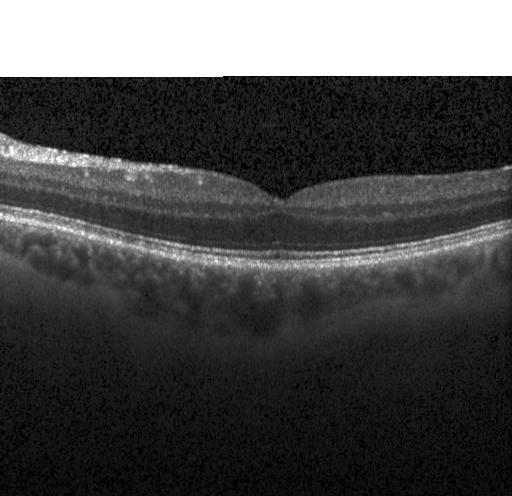 OCT line scan · acquired on a Heidelberg Spectralis.
Diagnosis: no evidence of choroidal neovascularization, diabetic macular edema, or drusen.